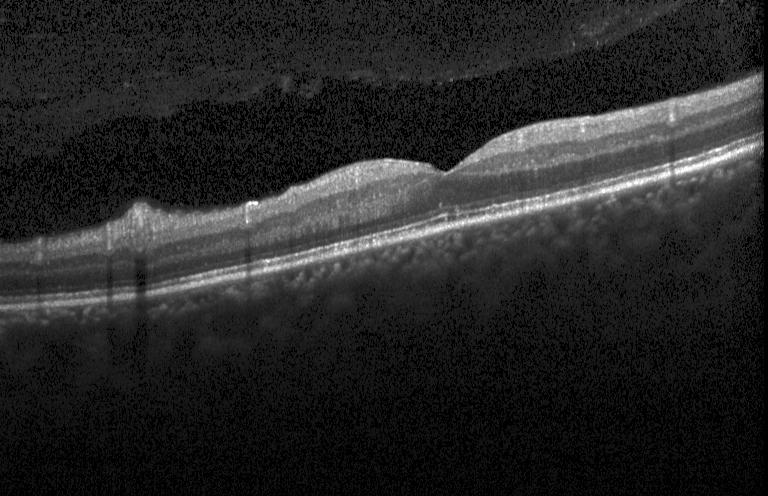
Impression: no choroidal neovascularization, no diabetic macular edema, and no drusen.